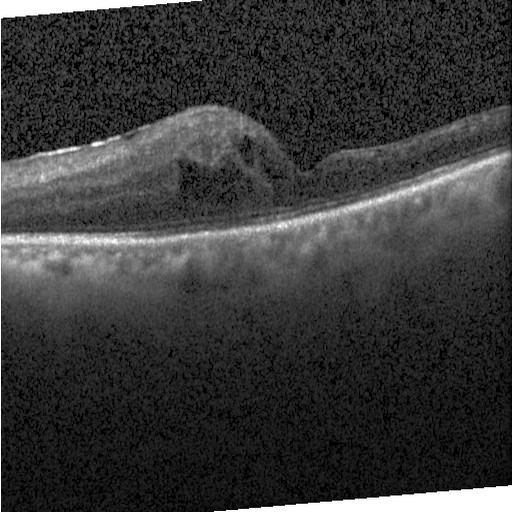

Spectral-domain OCT. Horizontal scan through the fovea. Retinal OCT B-scan. Instrument: Heidelberg Spectralis
Assessment: diabetic macular edema (DME).